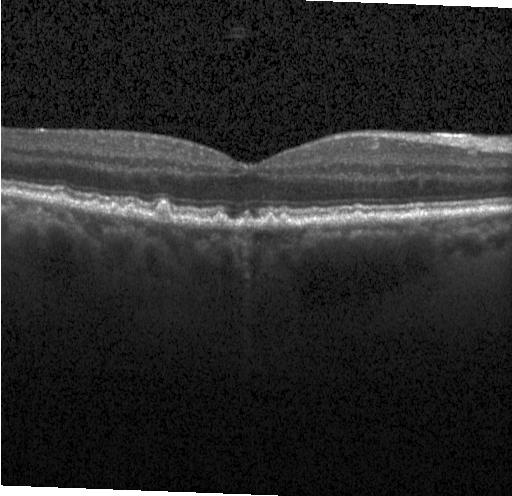
Acquired on a Heidelberg Spectralis. Retinal OCT B-scan — Macular OCT: multiple drusen.